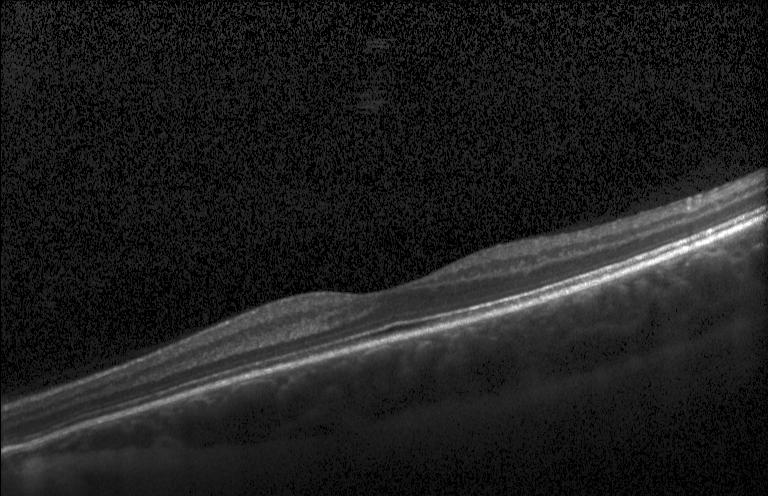 SD-OCT; retinal OCT cross-section
Assessment: no CNV, no DME, and no drusen.